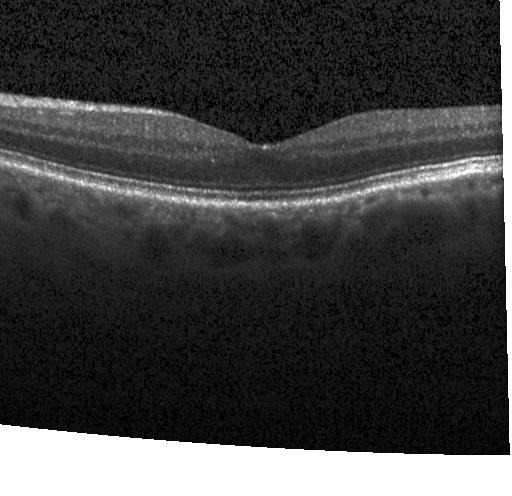

OCT B-scan. Spectral-domain optical coherence tomography. Heidelberg Spectralis OCT system.
Finding: no evidence of choroidal neovascularization, diabetic macular edema, or drusen.